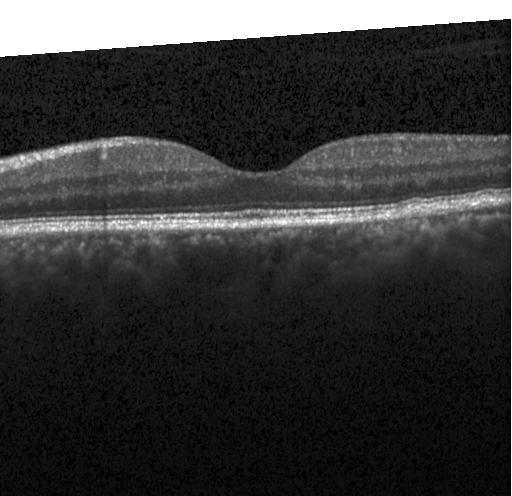 Optical coherence tomography scan
No CNV, DME, or drusen.